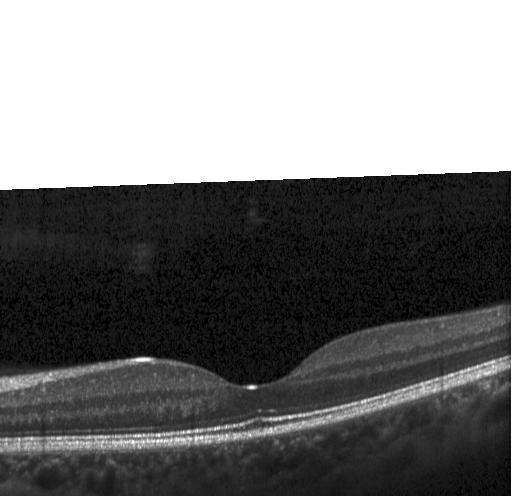

Macular OCT demonstrating no choroidal neovascularization, no diabetic macular edema, and no drusen.